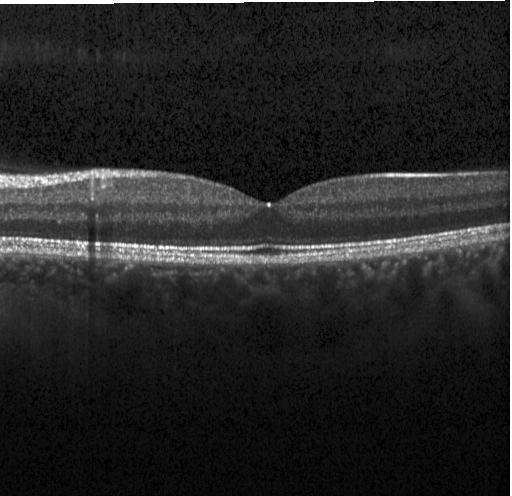 Retinal OCT B-scan. Impression: neither choroidal neovascularization, diabetic macular edema, nor drusen.